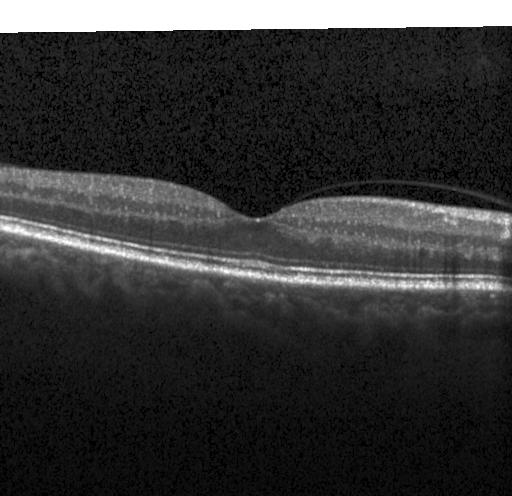

Spectral-domain OCT. Retinal OCT B-scan. Impression: no choroidal neovascularization, diabetic macular edema, or drusen.